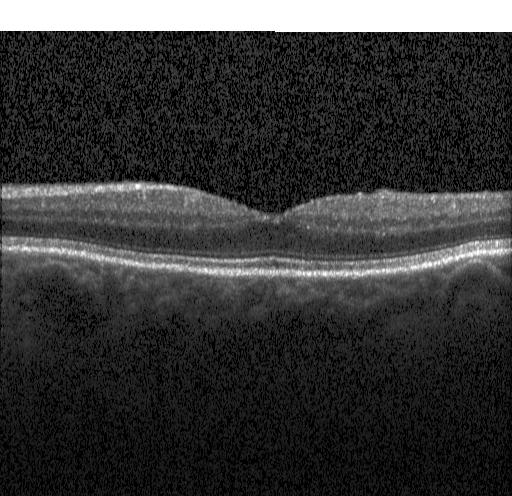

Finding: no CNV, no DME, and no drusen.